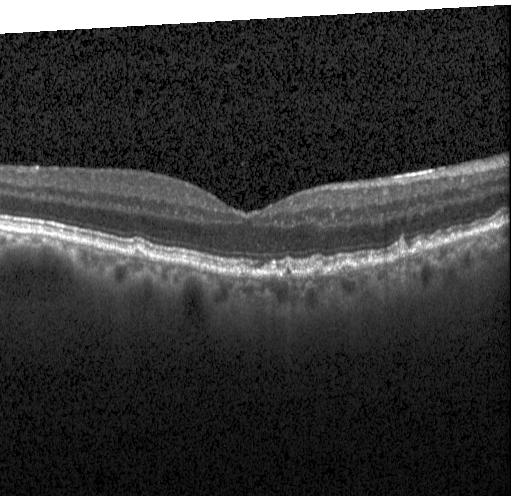 Acquired on a Heidelberg Spectralis · SD-OCT · optical coherence tomography scan · macular scan. Finding: sub-RPE drusenoid deposits.